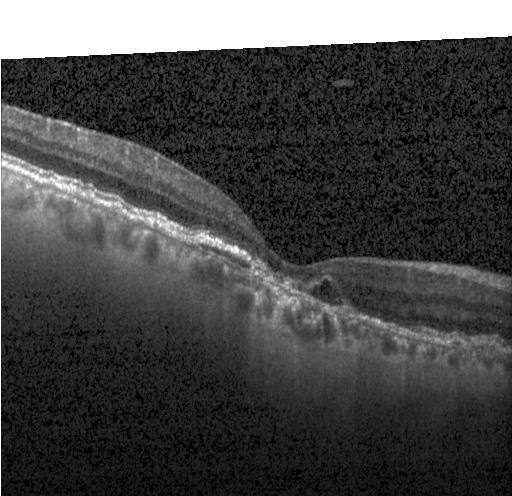 Retinal OCT cross-section showing choroidal neovascularization.